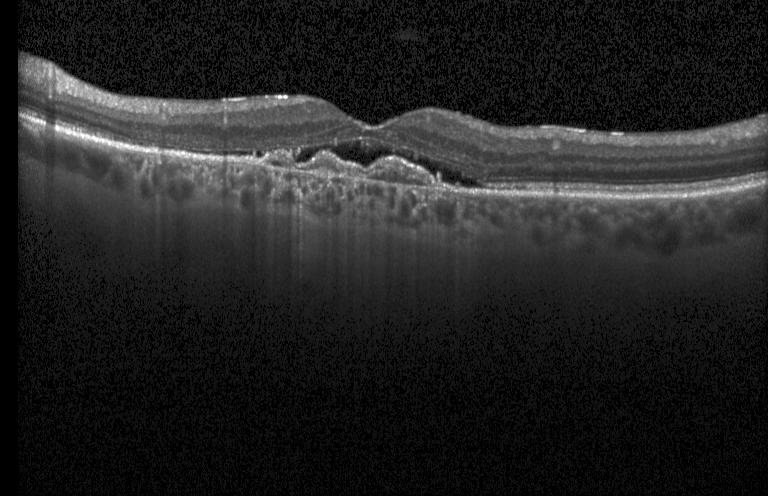 The scan shows a choroidal neovascular membrane.